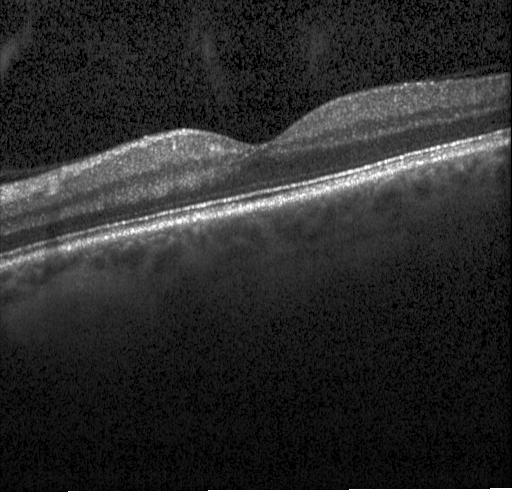
Retinal OCT cross-section showing no choroidal neovascularization, diabetic macular edema, or drusen.